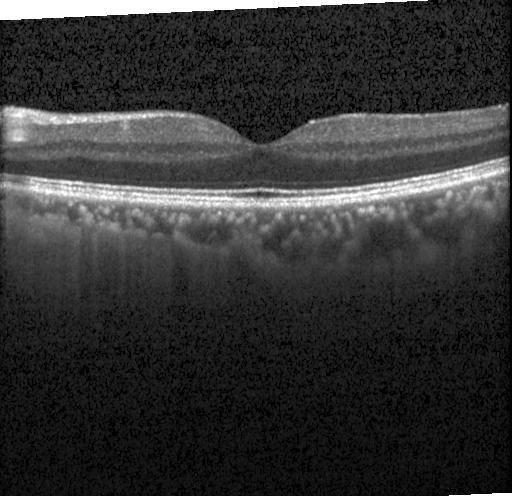
Dx: no CNV, no DME, and no drusen.